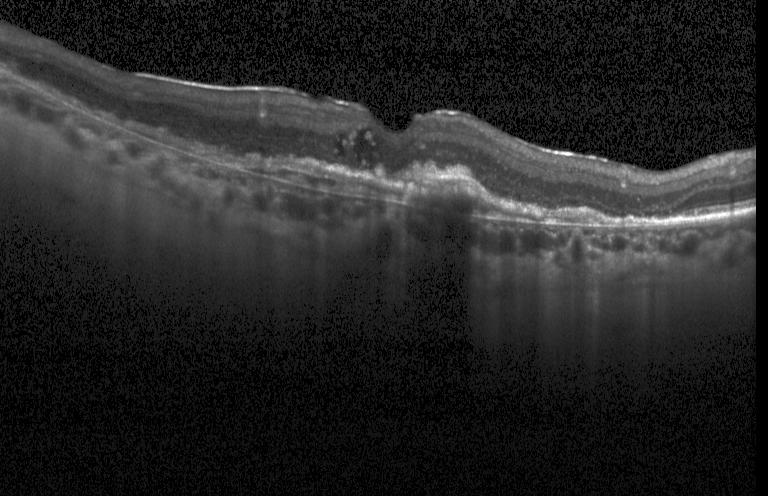
Diagnosis: a choroidal neovascular membrane.